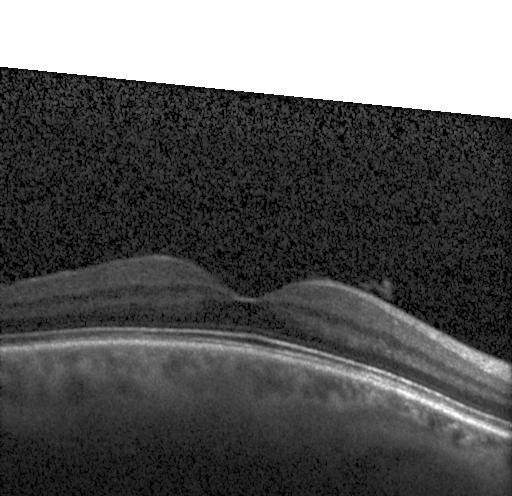

Finding: no evidence of choroidal neovascularization, diabetic macular edema, or drusen.